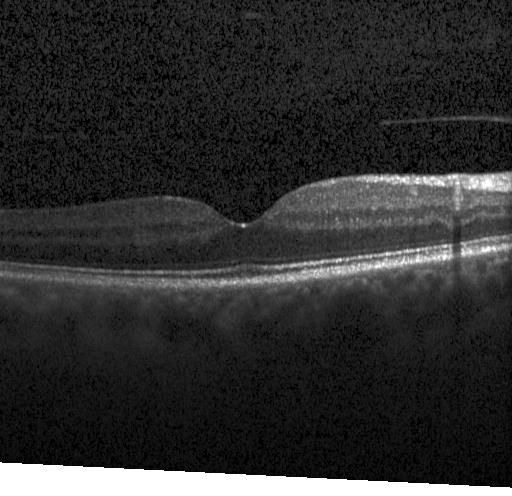

Through the macula, optical coherence tomography B-scan, spectral-domain optical coherence tomography, Heidelberg Spectralis OCT system
Neither choroidal neovascularization, diabetic macular edema, nor drusen.